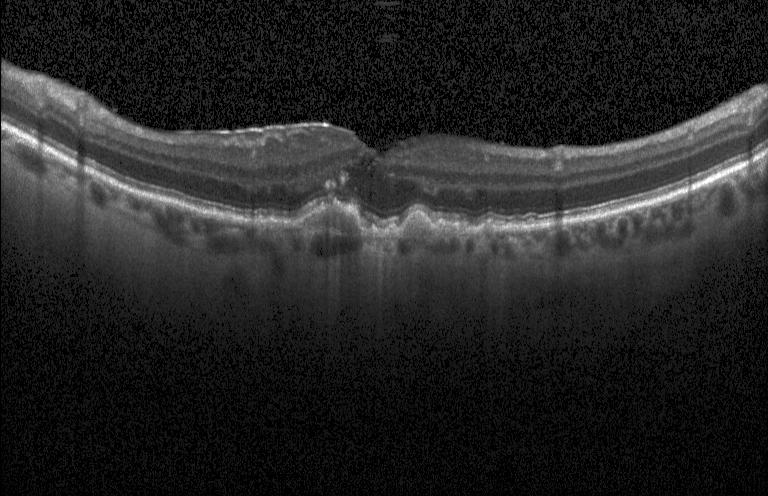 Dx: a choroidal neovascular membrane.